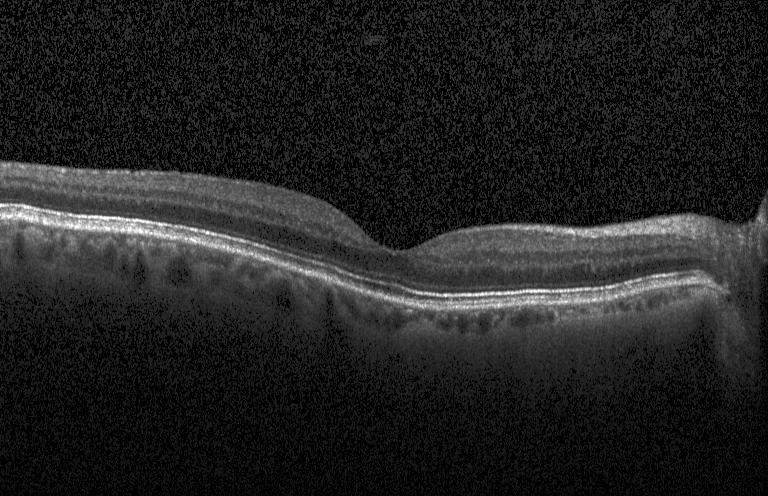

Optical coherence tomography B-scan; SD-OCT
Dx: no choroidal neovascularization, diabetic macular edema, or drusen.